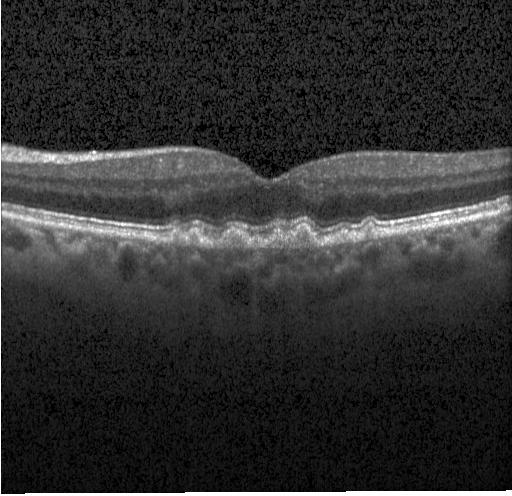 OCT B-scan showing drusen.